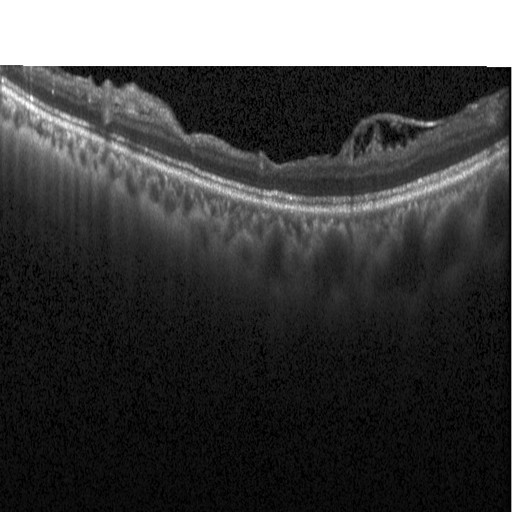

Retinal OCT B-scan · macular scan · spectral-domain OCT · Heidelberg Spectralis OCT system.
Finding: diabetic macular edema (DME).